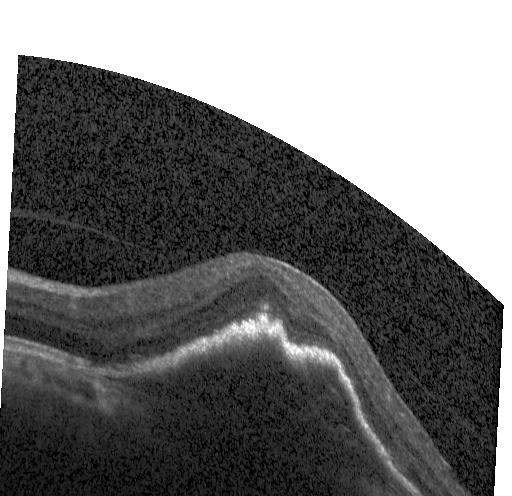
OCT line scan; spectral-domain optical coherence tomography; instrument: Heidelberg Spectralis; fovea-centered. Macular OCT: a choroidal neovascular membrane.